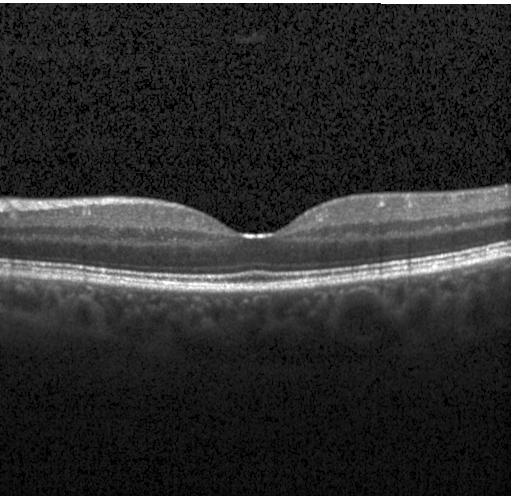

No CNV, DME, or drusen.